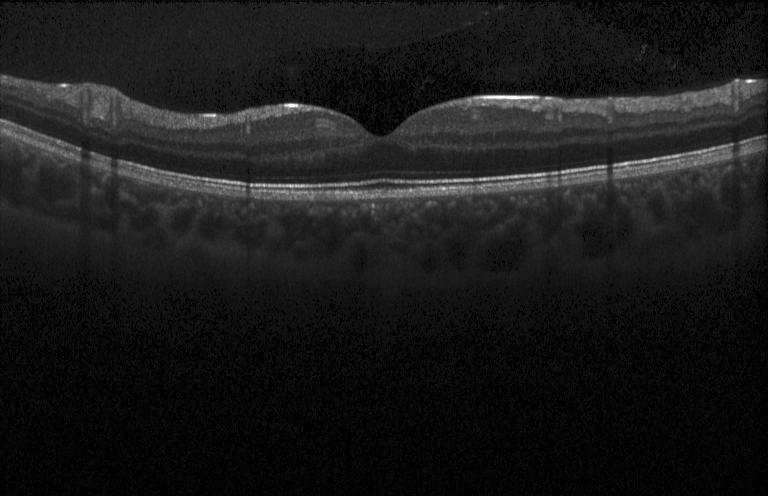

Heidelberg Spectralis · retinal OCT cross-section.
Finding: no choroidal neovascularization, diabetic macular edema, or drusen.